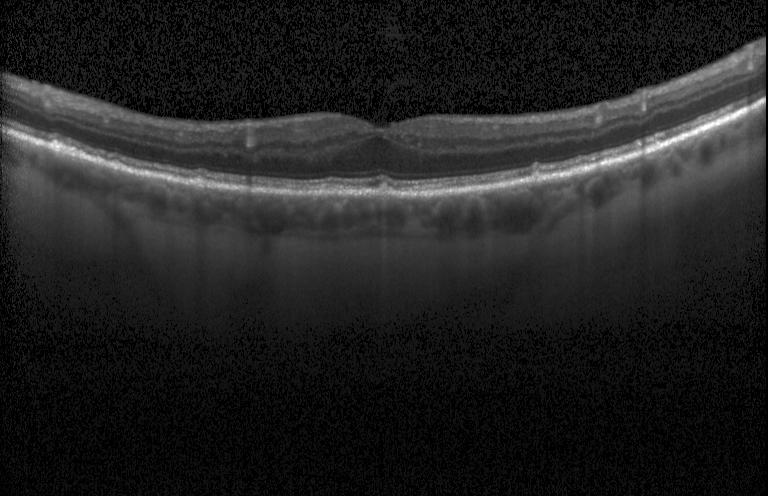

Macular scan, OCT B-scan, spectral-domain OCT, Heidelberg Spectralis — Sub-RPE drusenoid deposits.